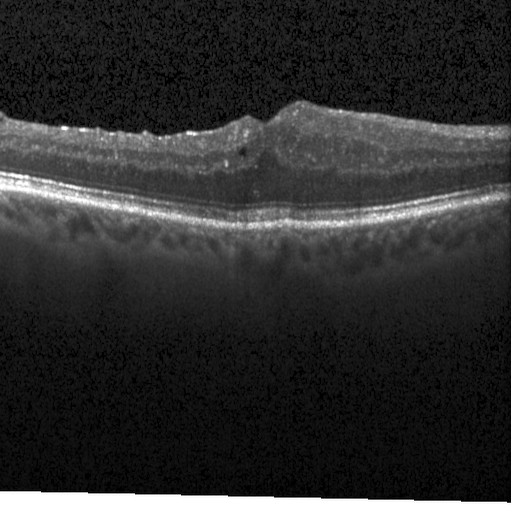 Retinal OCT cross-section showing diabetic macular edema.